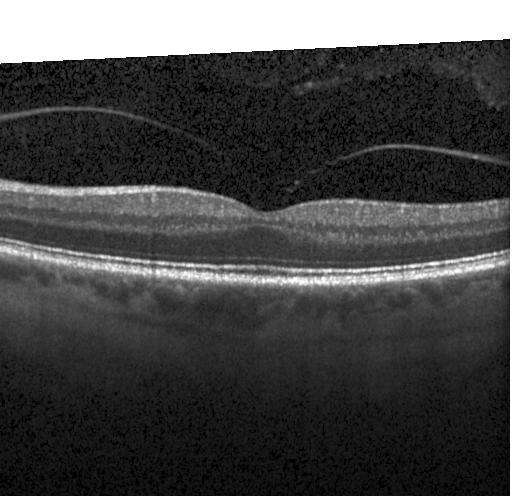

Optical coherence tomography B-scan; spectral-domain optical coherence tomography.
Diagnosis: no choroidal neovascularization, diabetic macular edema, or drusen.